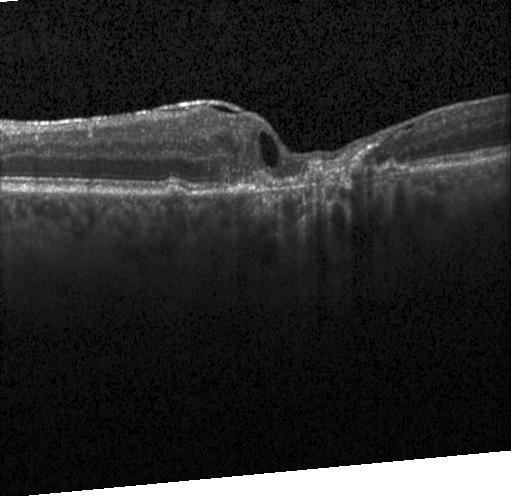
Diagnosis: CNV.